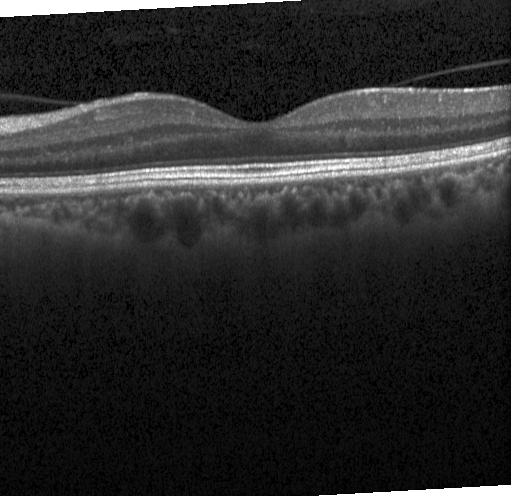 Spectral-domain optical coherence tomography; through the macula; retinal OCT B-scan
Diagnosis: no choroidal neovascularization, no diabetic macular edema, and no drusen.